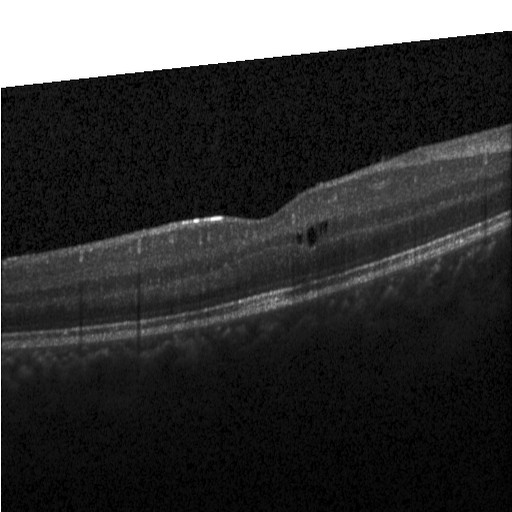

Optical coherence tomography B-scan
The scan shows diabetic macular edema.